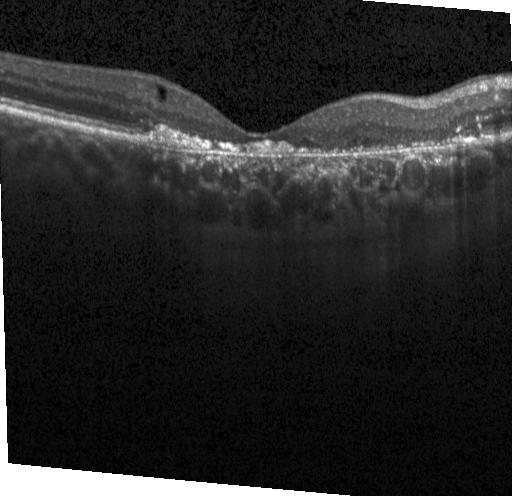

OCT B-scan. OCT finding: choroidal neovascularization.